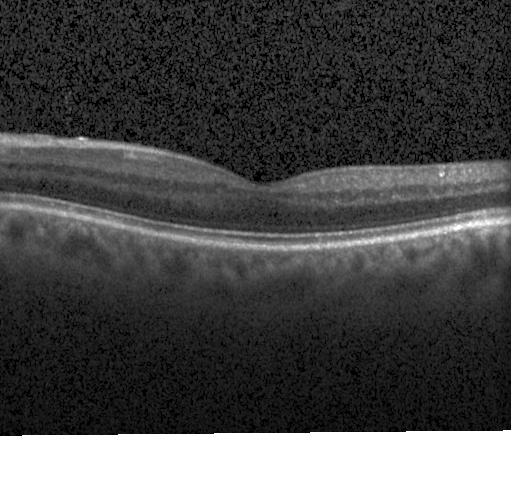
Diagnosis: no CNV, no DME, and no drusen.